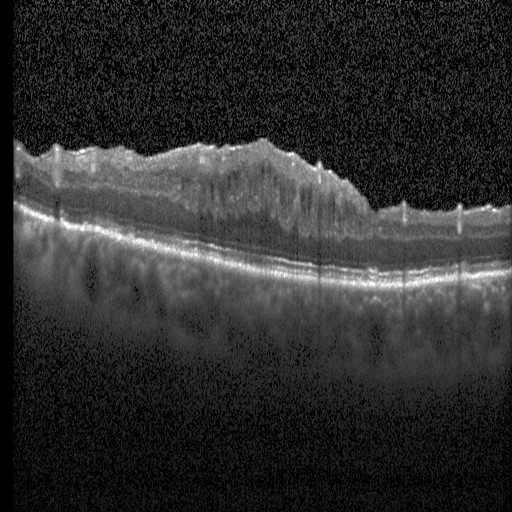

Dx: diabetic macular edema (DME).